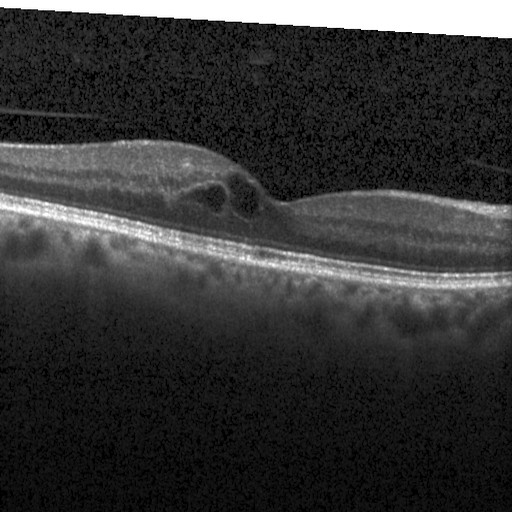
Optical coherence tomography scan; fovea-centered; SD-OCT.
The scan shows diabetic macular edema (DME).